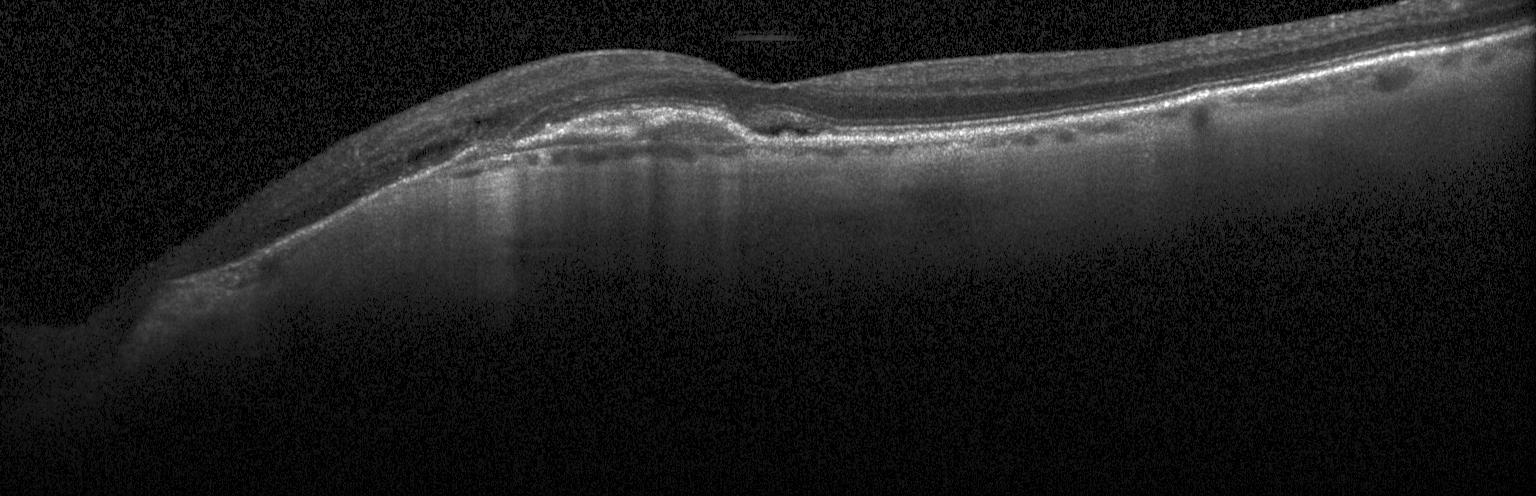

Impression: choroidal neovascularization (CNV).